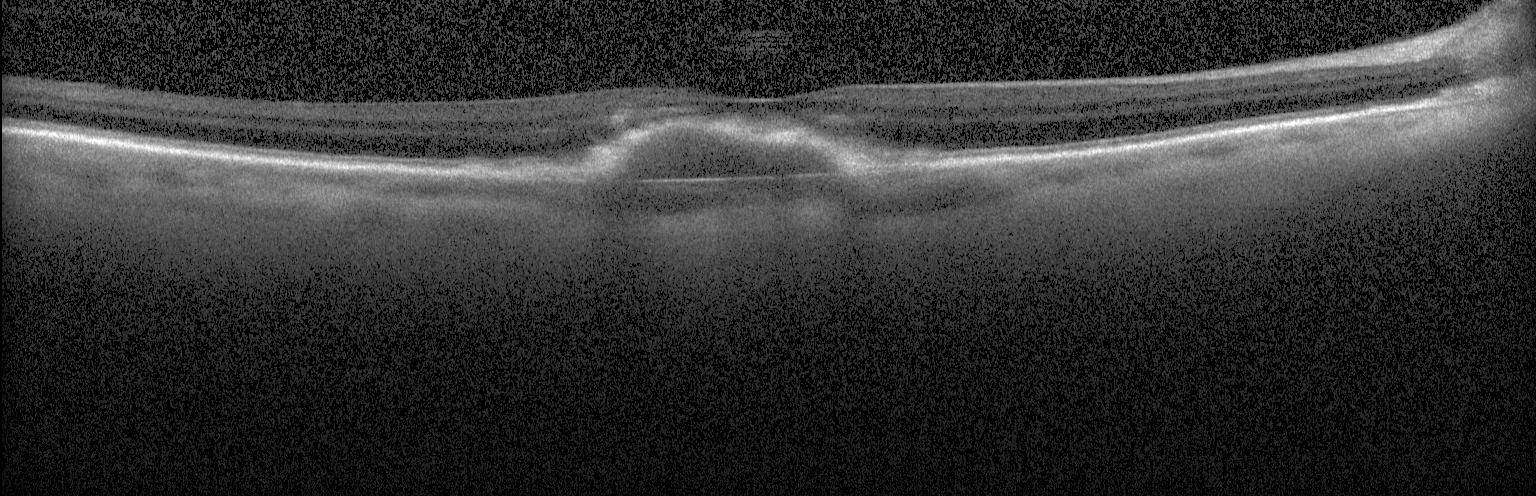
Impression: CNV.